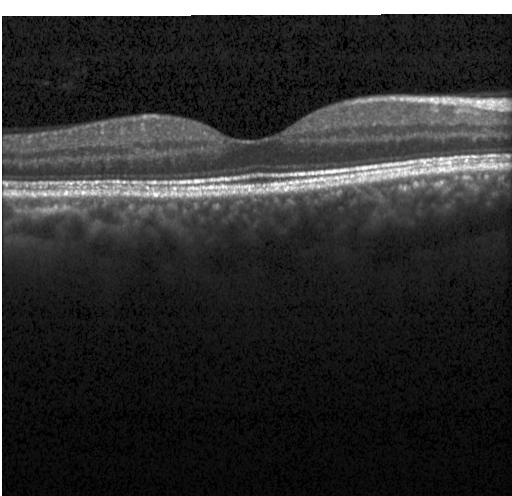

Dx: neither choroidal neovascularization, diabetic macular edema, nor drusen.